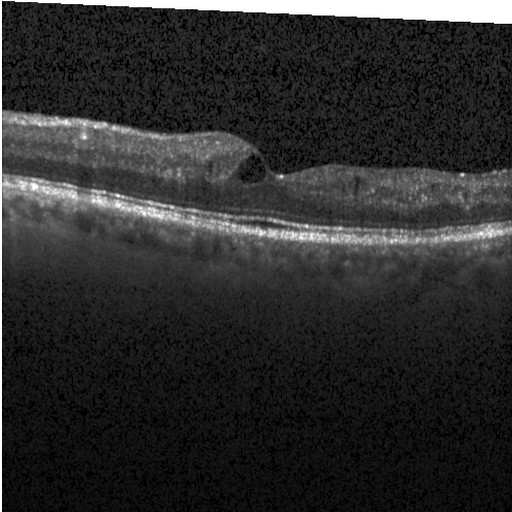
Heidelberg Spectralis, horizontal scan through the fovea, retinal OCT cross-section — Finding: diabetic macular edema (DME).